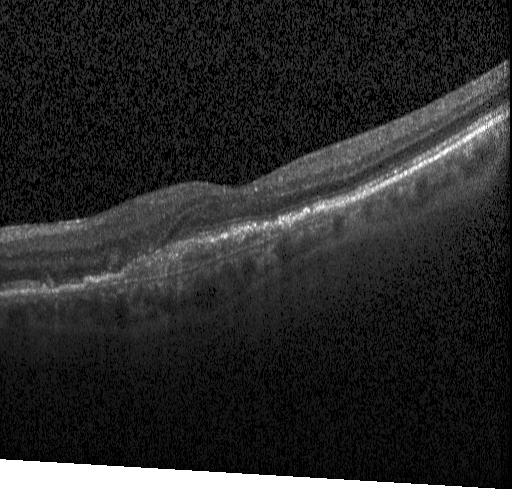
Macular OCT demonstrating a choroidal neovascular membrane.